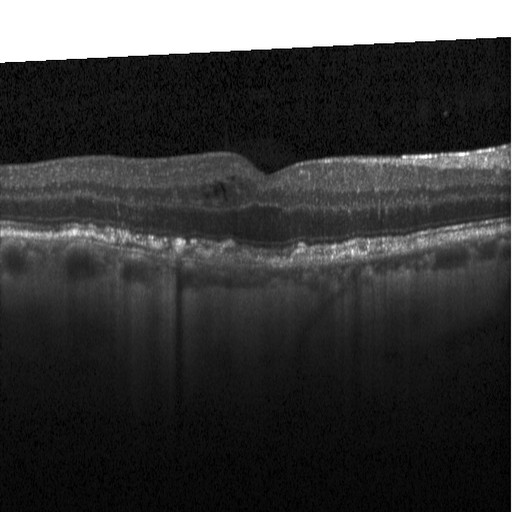
Finding: diabetic macular edema (DME).